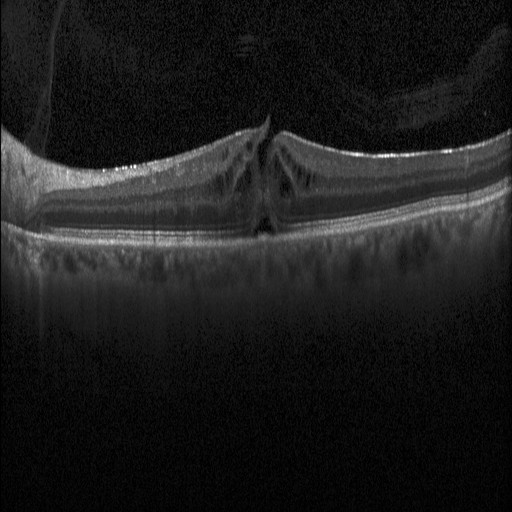

Spectral-domain OCT · retinal OCT B-scan — OCT finding: diabetic macular edema.